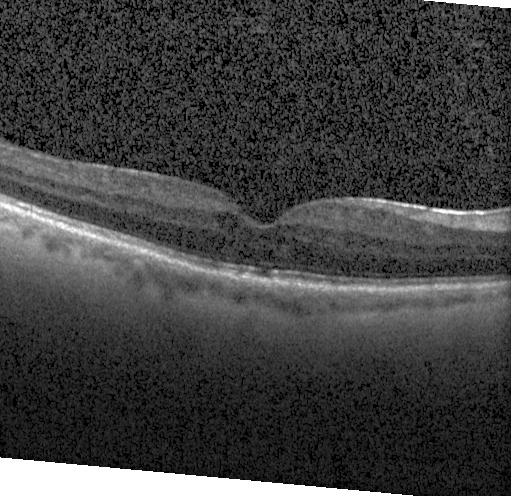
OCT scan showing no choroidal neovascularization, no diabetic macular edema, and no drusen.